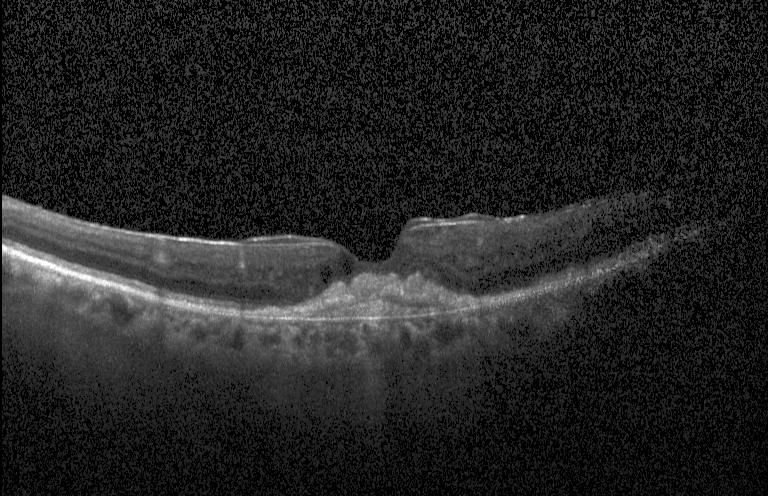 Diagnosis: choroidal neovascularization.